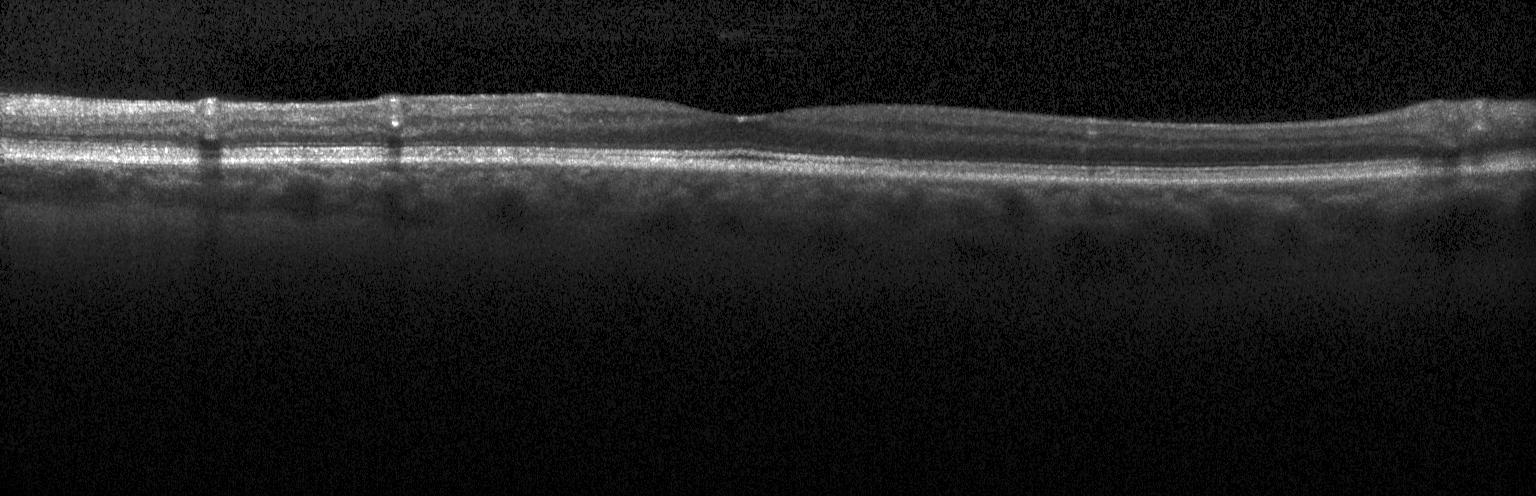

Finding: no choroidal neovascularization, no diabetic macular edema, and no drusen.